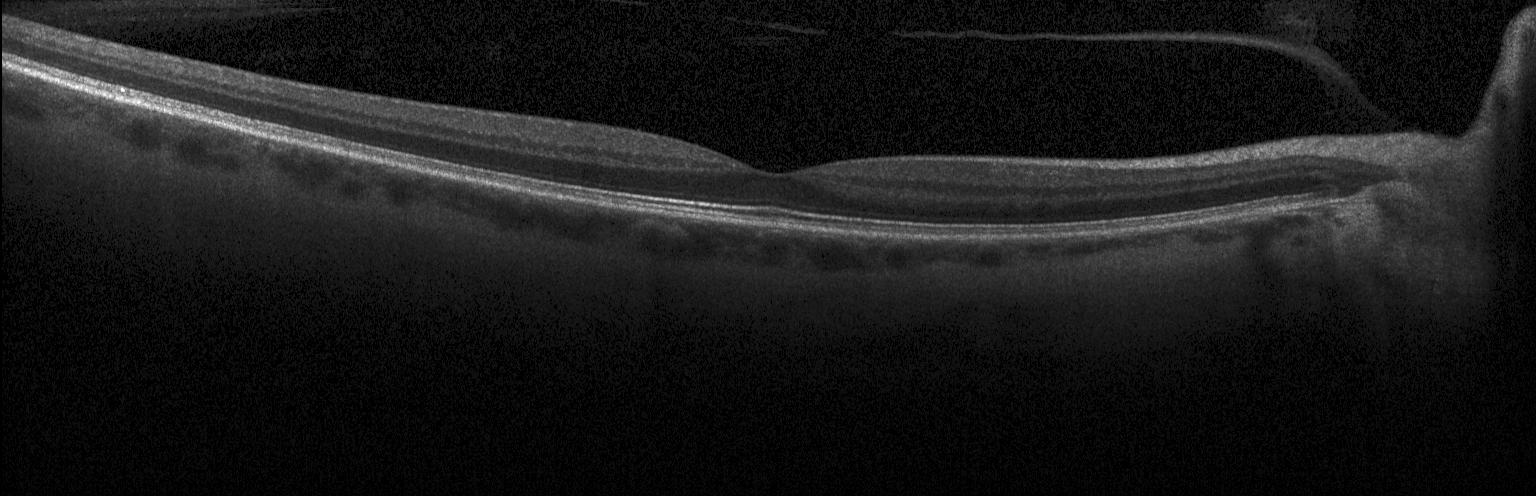
Retinal OCT cross-section; SD-OCT
This B-scan demonstrates no choroidal neovascularization, diabetic macular edema, or drusen.